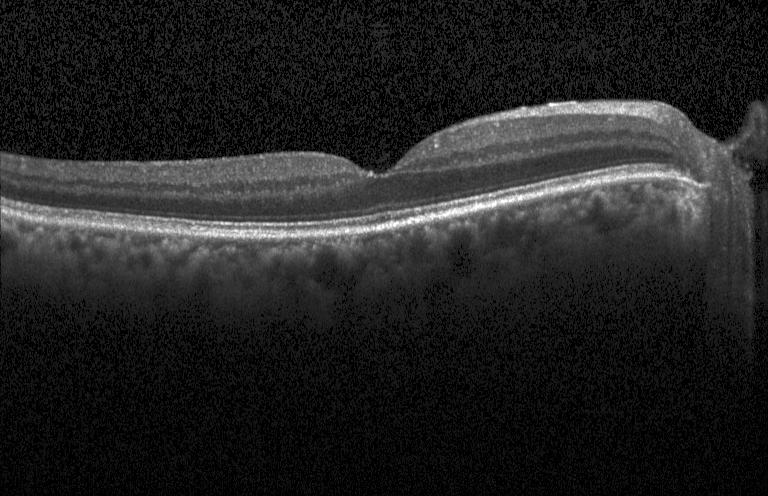

Retinal OCT cross-section; fovea-centered — This B-scan demonstrates no CNV, no DME, and no drusen.